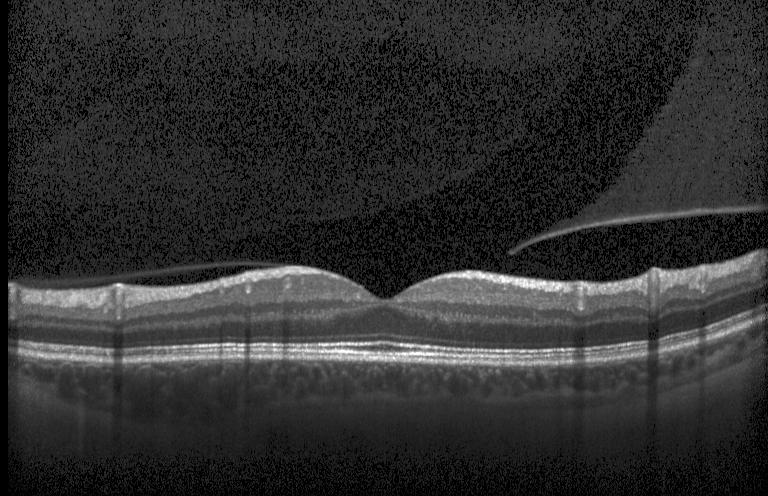

Neither choroidal neovascularization, diabetic macular edema, nor drusen.